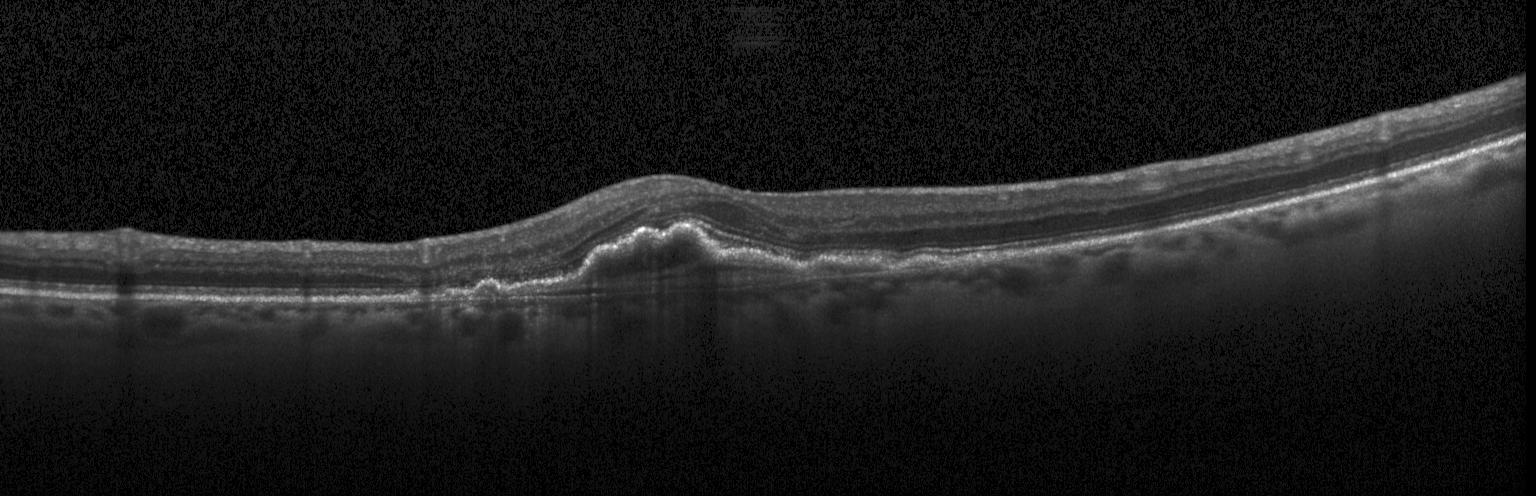
Spectral-domain OCT. OCT line scan. Instrument: Heidelberg Spectralis — This B-scan demonstrates a choroidal neovascular membrane.